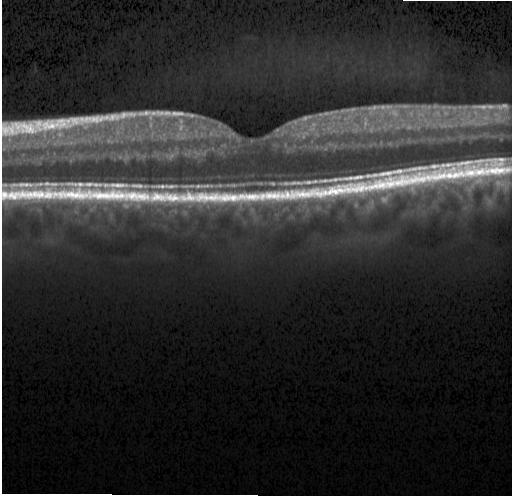 Retinal OCT B-scan · Heidelberg Spectralis OCT system
Dx: no evidence of choroidal neovascularization, diabetic macular edema, or drusen.